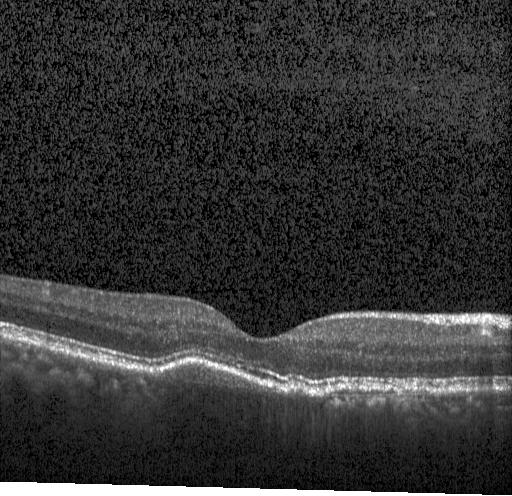
Retinal OCT cross-section, horizontal scan through the fovea.
Finding: multiple drusen.